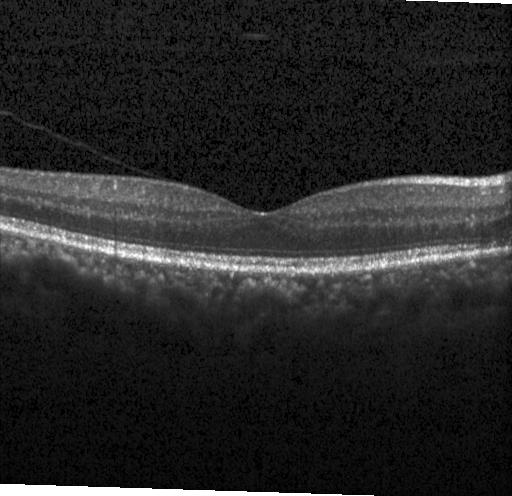

Impression: no CNV, no DME, and no drusen.